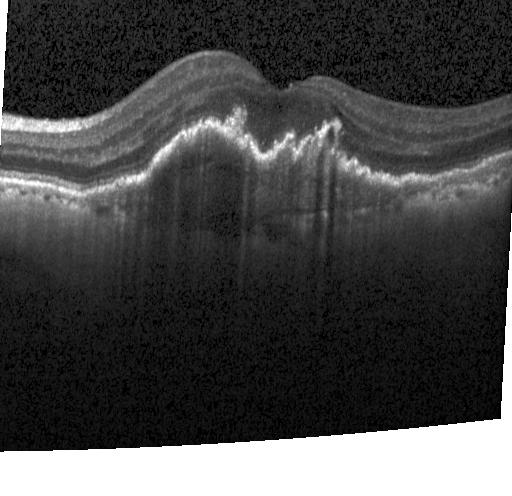

Diagnosis: a choroidal neovascular membrane.